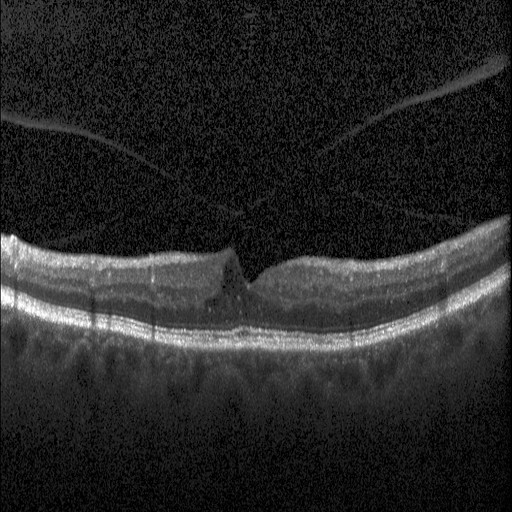

Impression: DME.